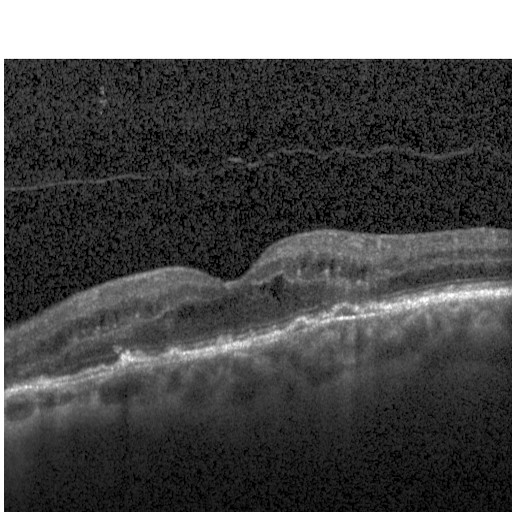 Horizontal scan through the fovea. Heidelberg Spectralis. OCT line scan — Finding: diabetic macular edema.